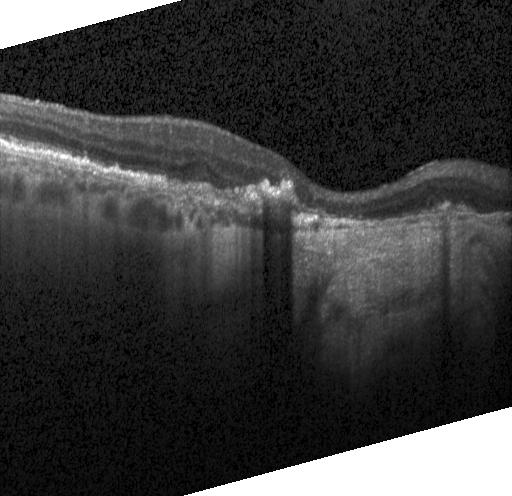 Diagnosis: a choroidal neovascular membrane.